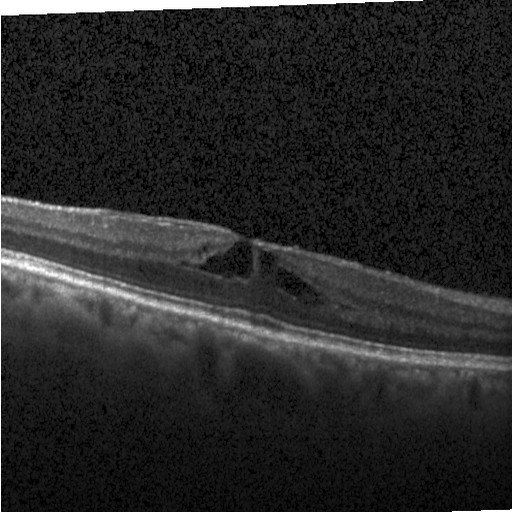 OCT B-scan
The scan shows DME.